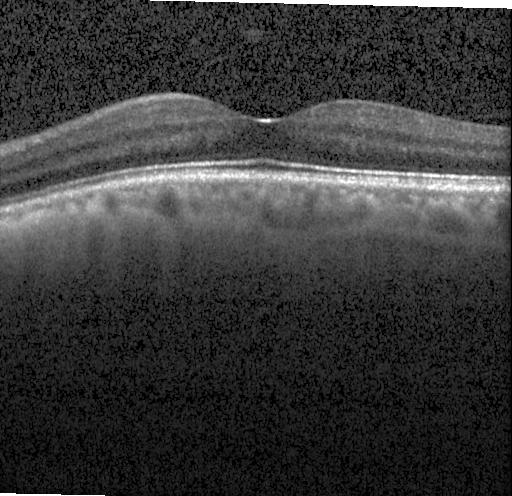
Diagnosis: no CNV, DME, or drusen.